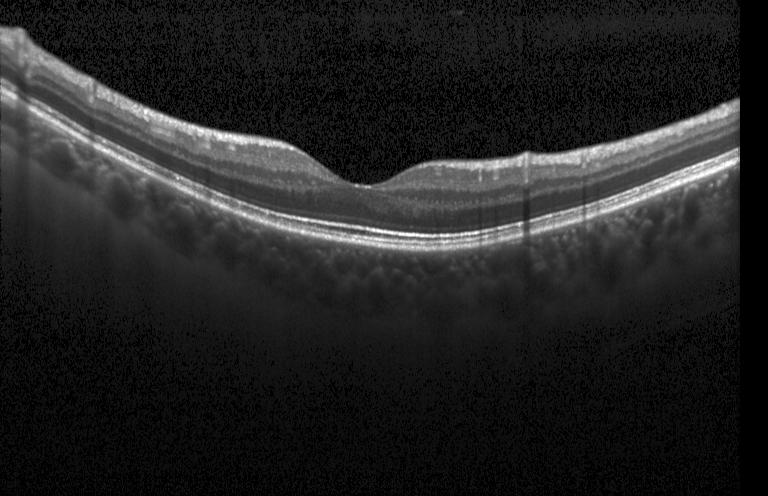

Macular OCT demonstrating no evidence of choroidal neovascularization, diabetic macular edema, or drusen.